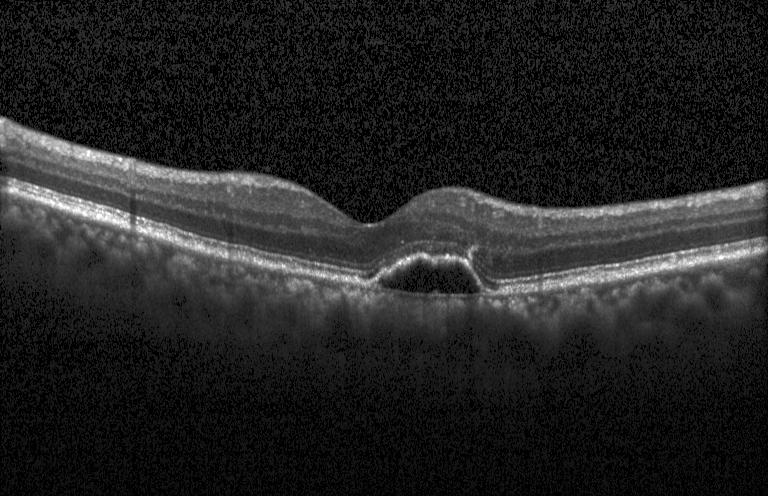 Dx: choroidal neovascularization (CNV).